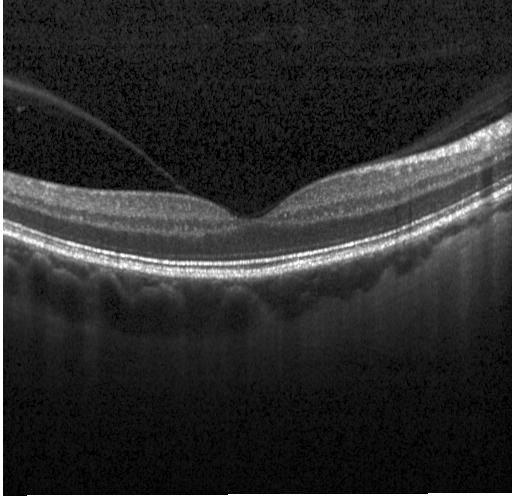
Retinal OCT cross-section.
Impression: neither choroidal neovascularization, diabetic macular edema, nor drusen.